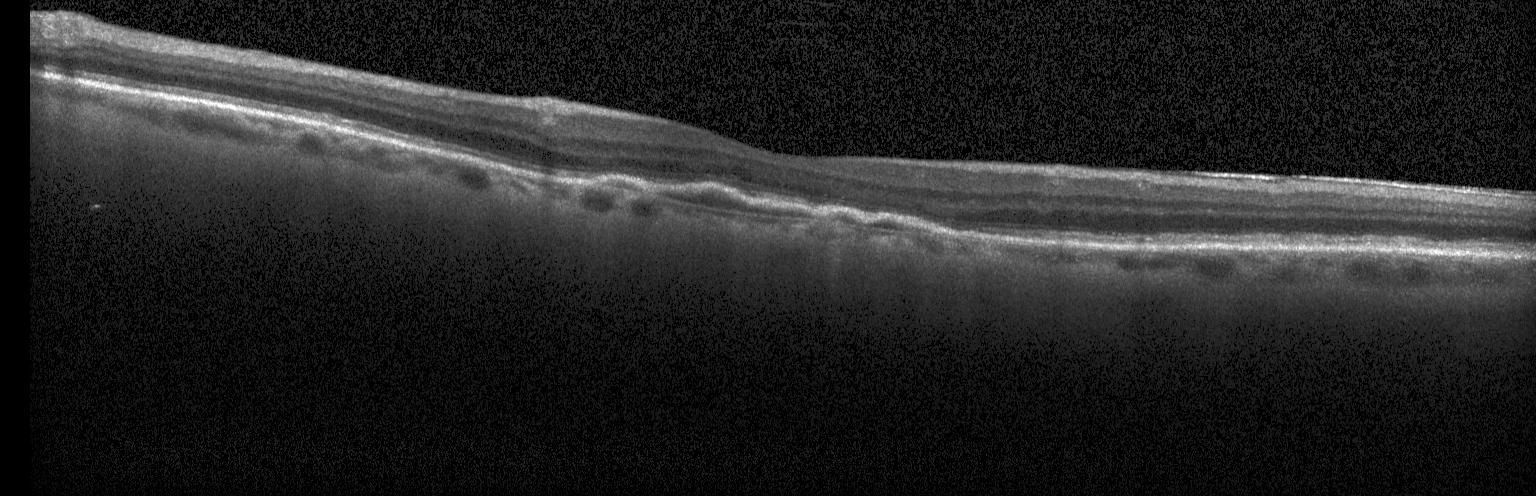
OCT B-scan showing a choroidal neovascular membrane.